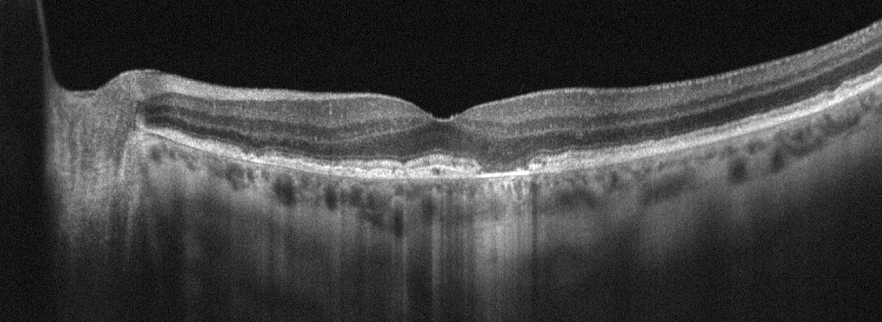
Fovea-centered. Retinal OCT B-scan
Finding: age-related macular degeneration.